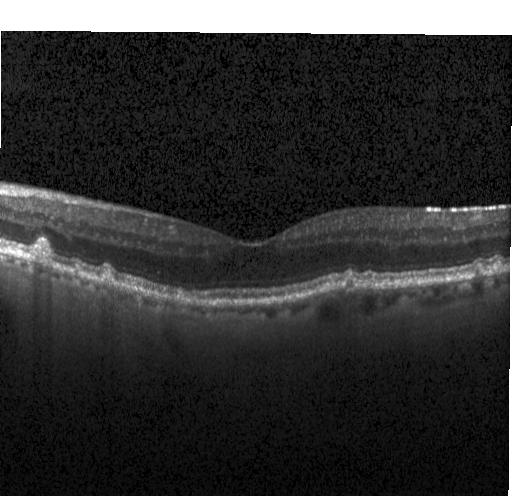

Dx: multiple drusen.